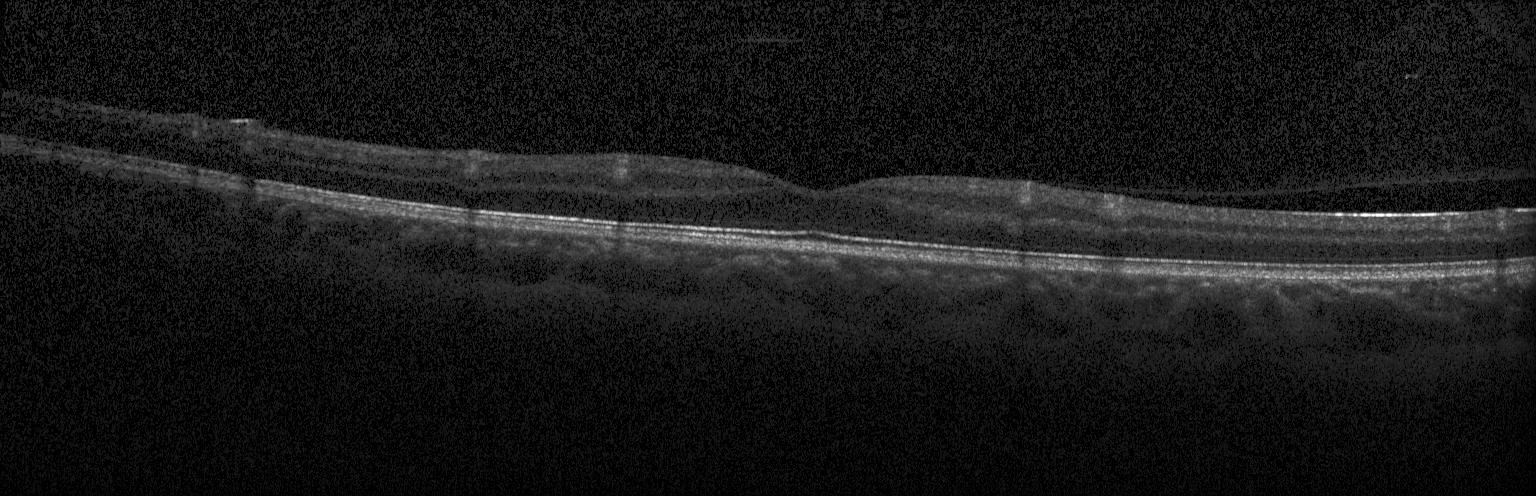 Optical coherence tomography B-scan. Assessment: neither choroidal neovascularization, diabetic macular edema, nor drusen.